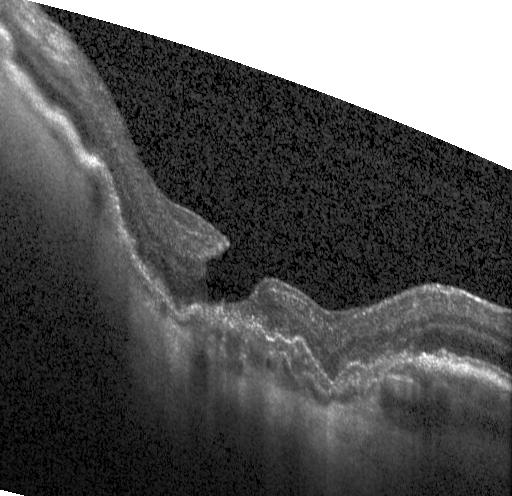 Dx: a choroidal neovascular membrane.